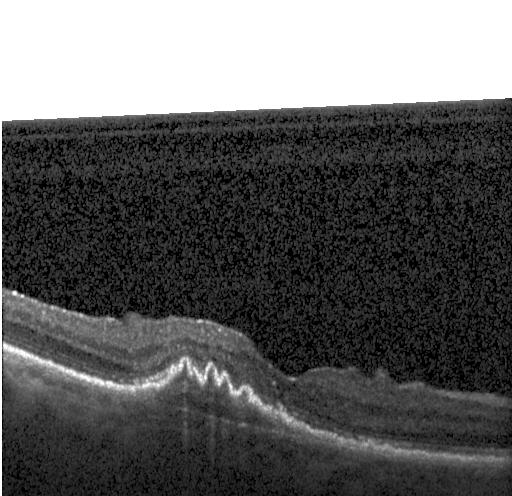 Instrument: Heidelberg Spectralis · OCT line scan · fovea-centered.
Diagnosis: CNV.